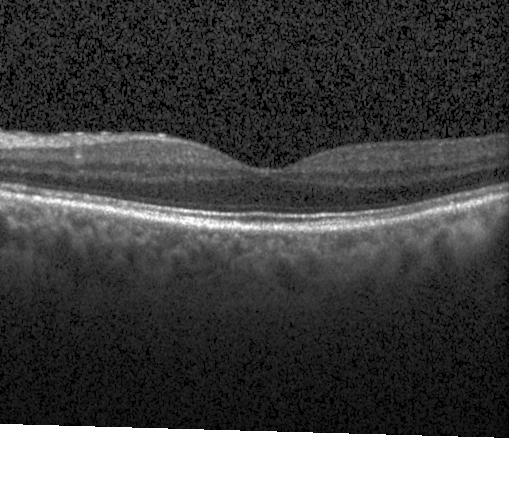
Retinal OCT cross-section showing no evidence of choroidal neovascularization, diabetic macular edema, or drusen.